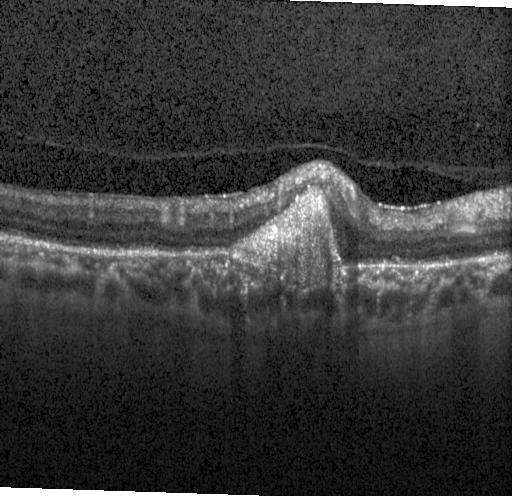
The scan shows a choroidal neovascular membrane.